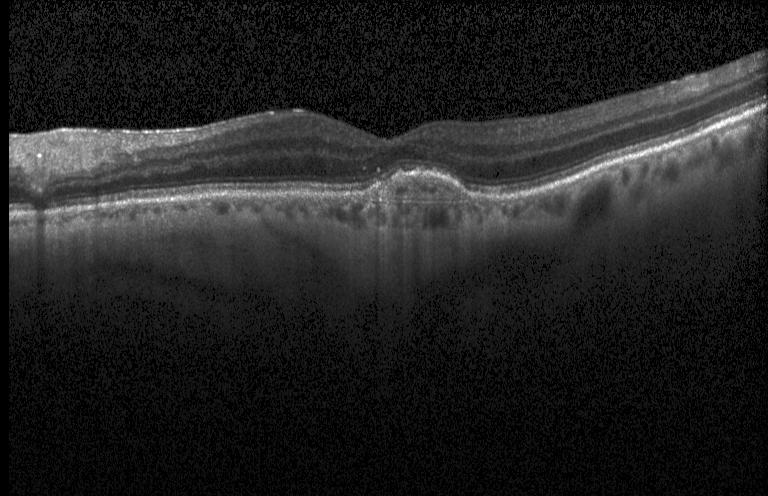 OCT B-scan · horizontal scan through the fovea. OCT finding: CNV.